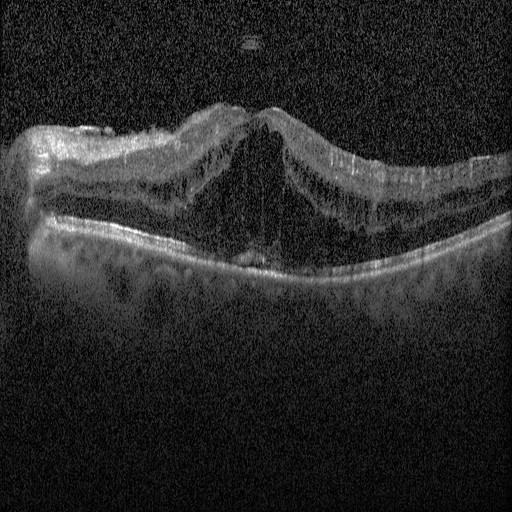 Finding: diabetic macular edema.